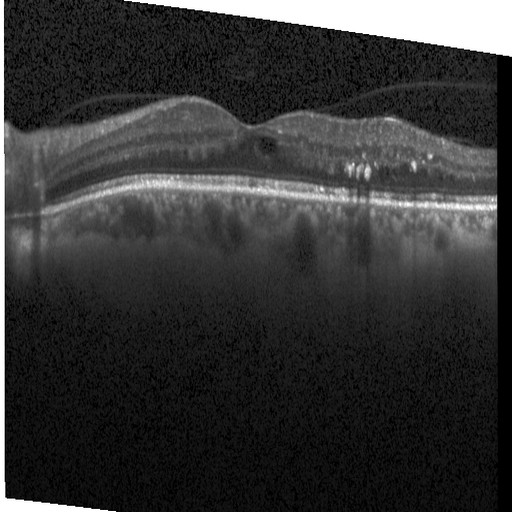
The scan shows DME.